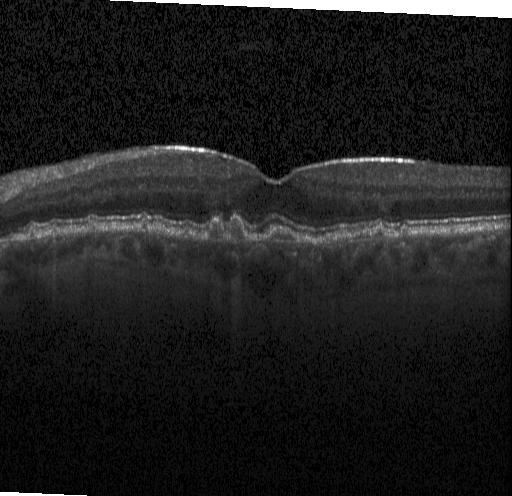

OCT B-scan; spectral-domain optical coherence tomography; horizontal scan through the fovea; instrument: Heidelberg Spectralis
OCT finding: multiple drusen.